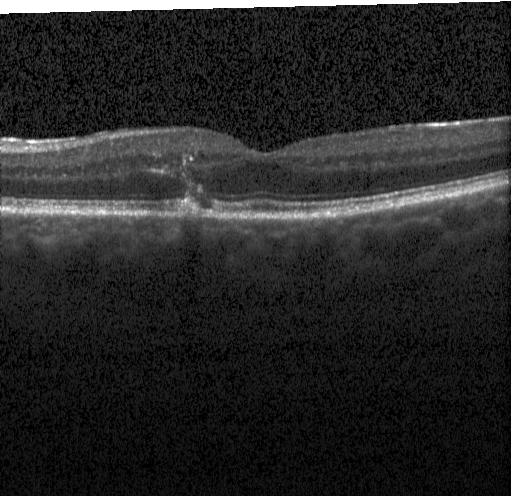

Optical coherence tomography B-scan — Diagnosis: choroidal neovascularization (CNV).